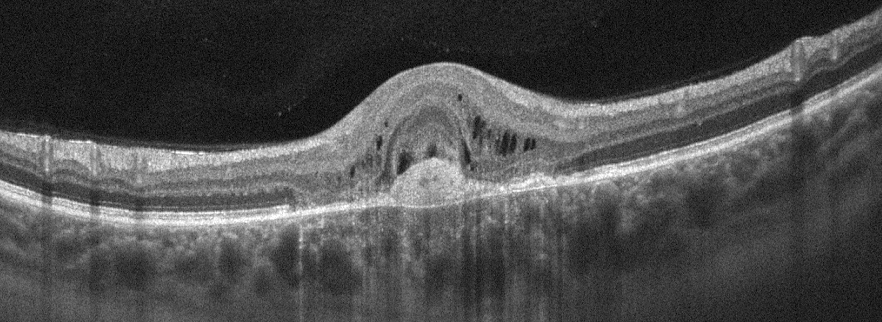 Optical coherence tomography scan · OD
Diagnosis: age-related macular degeneration (AMD).